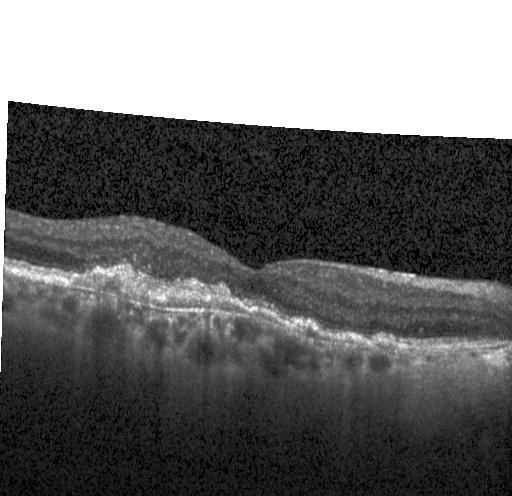
Impression: a choroidal neovascular membrane.